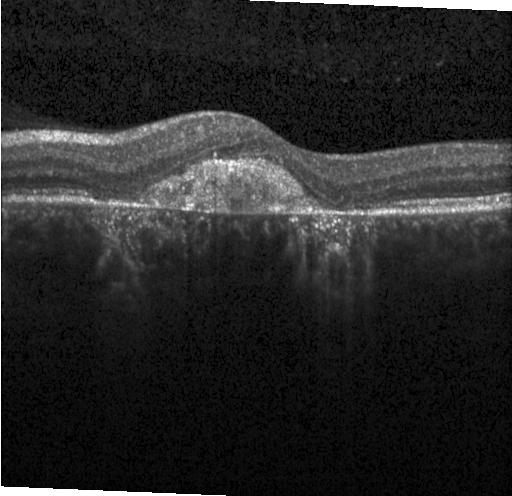
SD-OCT · retinal OCT cross-section. Finding: a choroidal neovascular membrane.